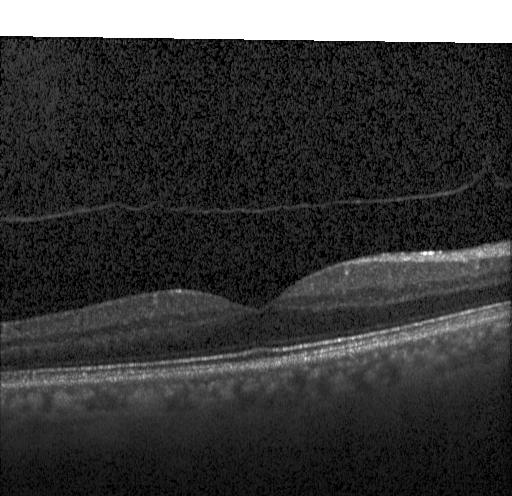 Retinal OCT B-scan; instrument: Heidelberg Spectralis.
Impression: no evidence of CNV, DME, or drusen.